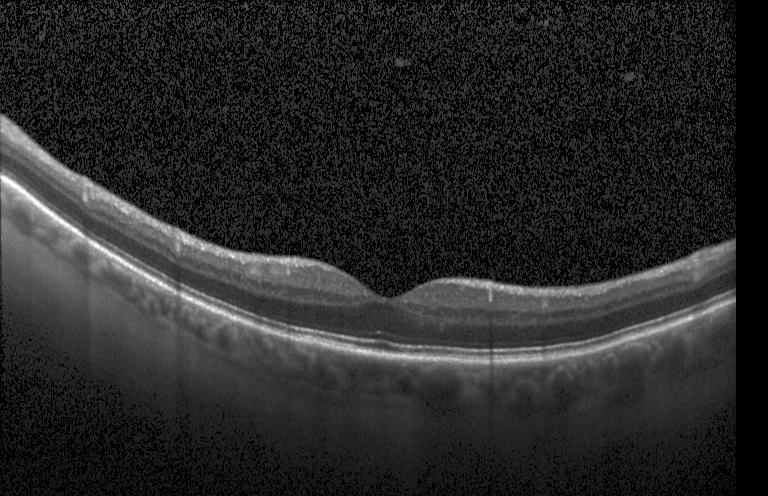 Finding: neither choroidal neovascularization, diabetic macular edema, nor drusen.